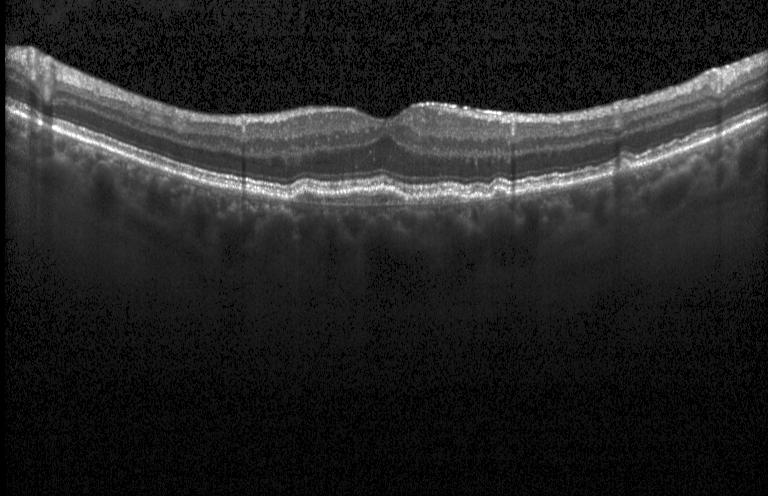 OCT B-scan showing choroidal neovascularization.